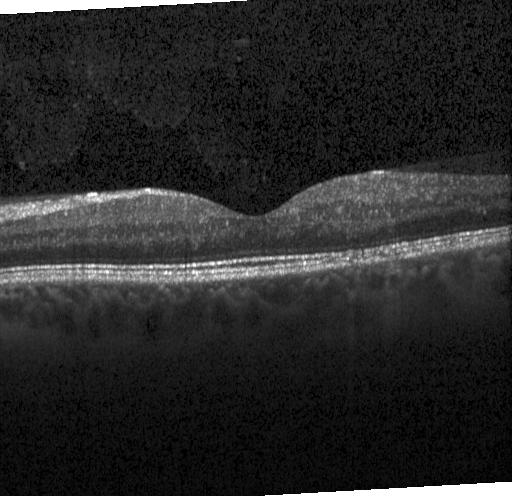
Finding: no choroidal neovascularization, diabetic macular edema, or drusen.